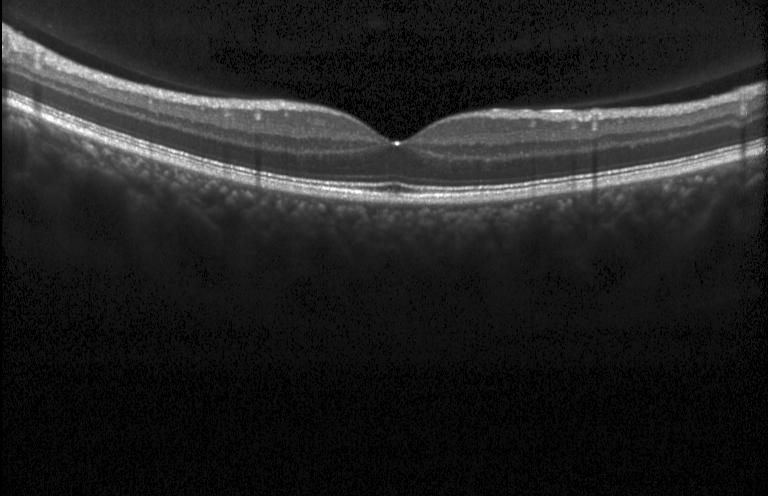
Finding: neither choroidal neovascularization, diabetic macular edema, nor drusen.